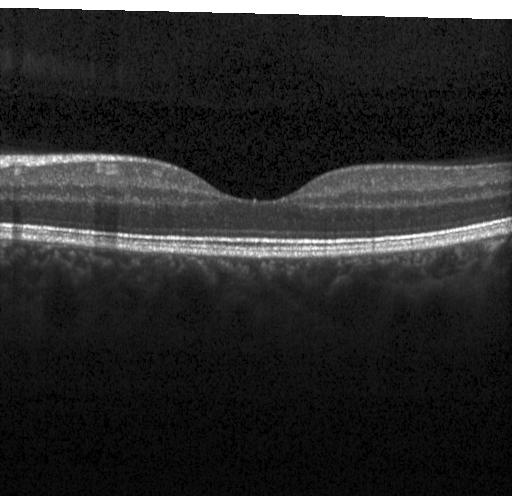 Fovea-centered; spectral-domain optical coherence tomography; Heidelberg Spectralis; retinal OCT cross-section — Impression: neither choroidal neovascularization, diabetic macular edema, nor drusen.